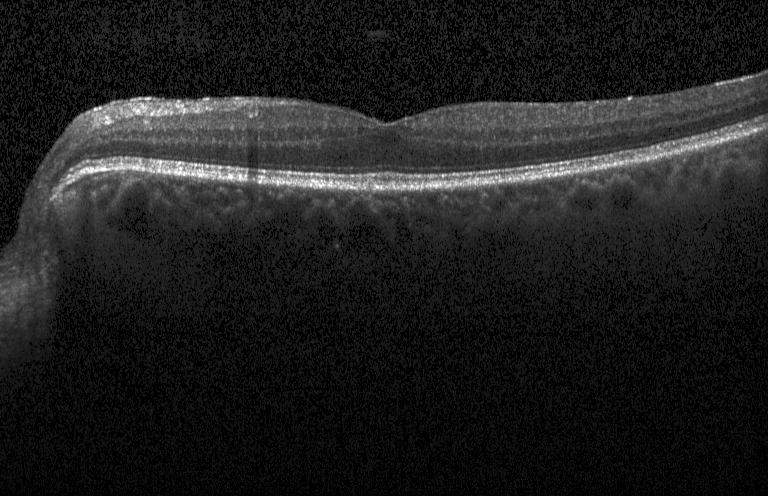

OCT B-scan showing no choroidal neovascularization, diabetic macular edema, or drusen.